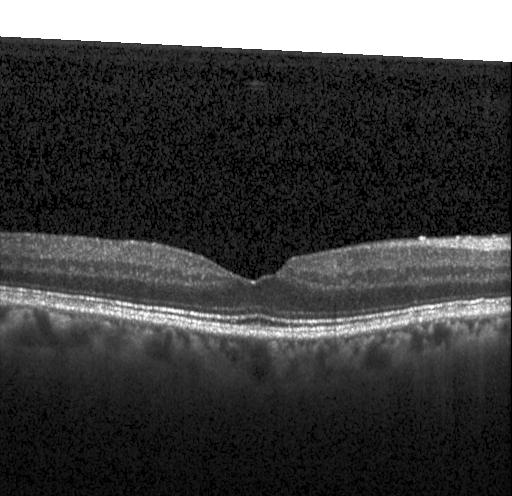

Acquired on a Heidelberg Spectralis. OCT B-scan. Horizontal scan through the fovea. SD-OCT — Assessment: no evidence of CNV, DME, or drusen.